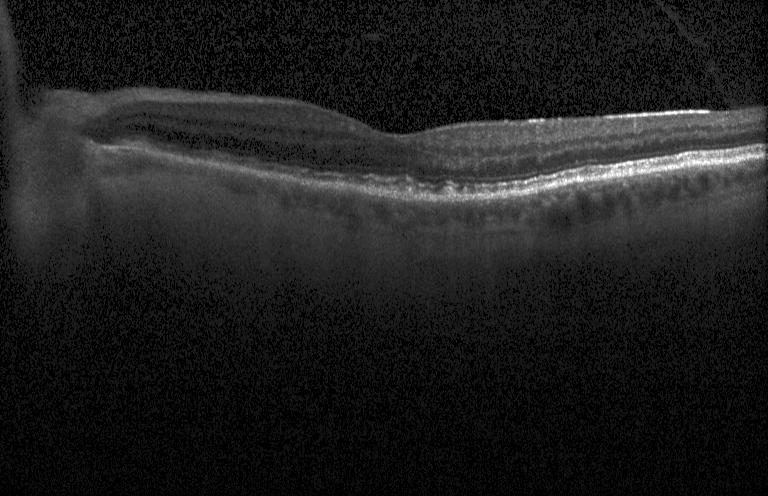

Spectral-domain OCT B-scan: drusen.